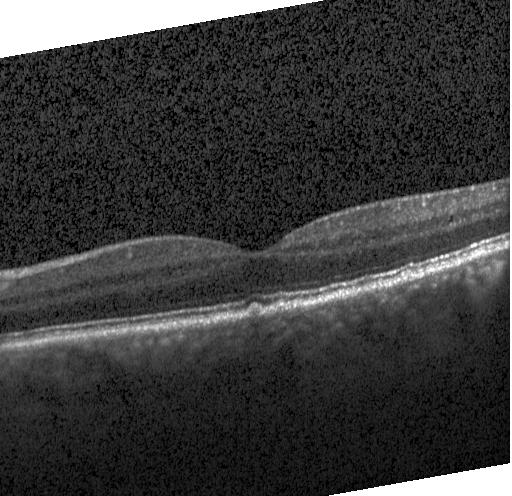

OCT B-scan showing multiple drusen.